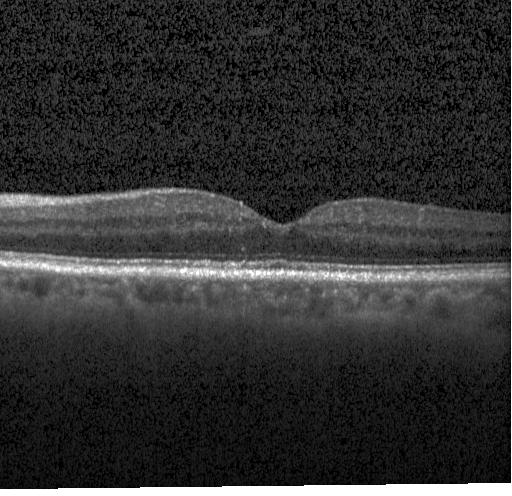

Finding: neither CNV, DME, nor drusen.